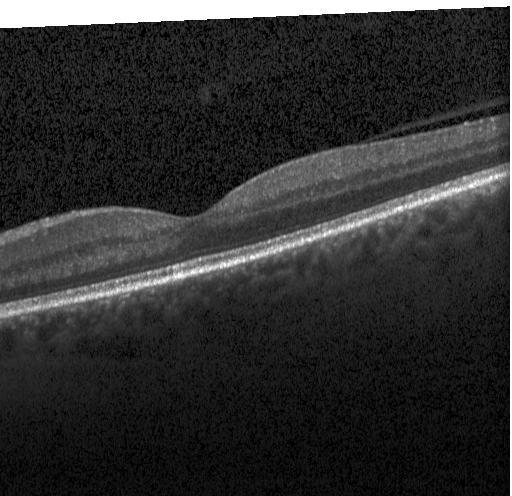 Instrument: Heidelberg Spectralis. Retinal OCT cross-section
No choroidal neovascularization, diabetic macular edema, or drusen.